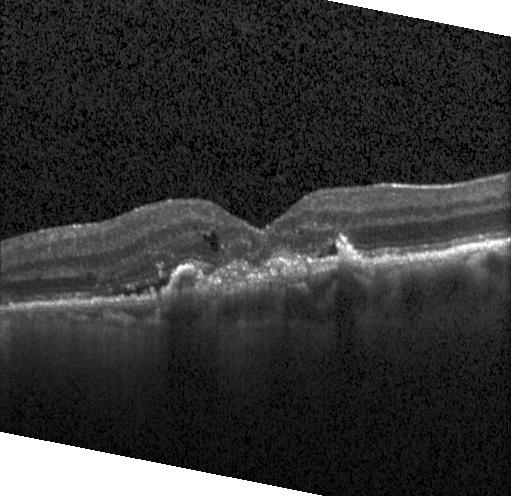

Optical coherence tomography B-scan. OCT finding: choroidal neovascularization.